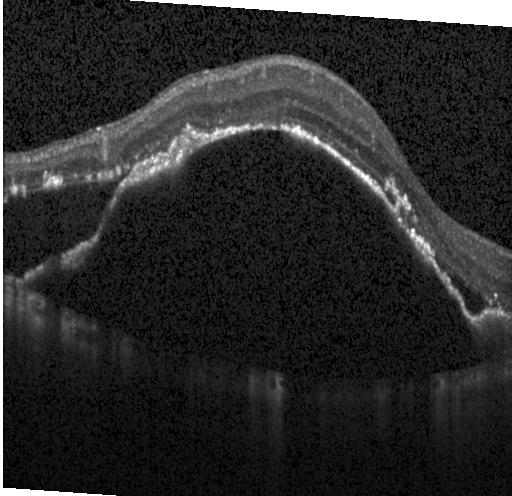

Retinal OCT B-scan.
The scan shows a choroidal neovascular membrane.